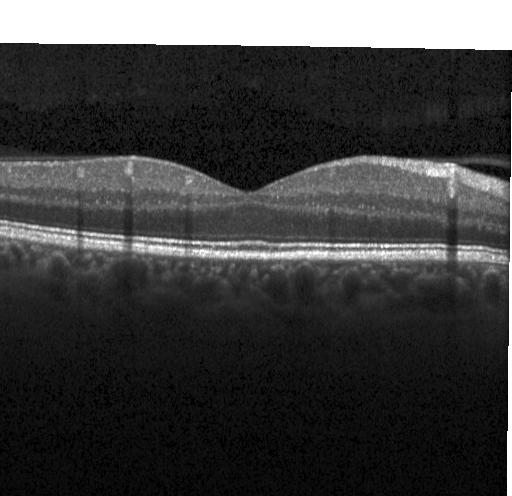
Optical coherence tomography scan · instrument: Heidelberg Spectralis · through the macula · spectral-domain OCT. Assessment: neither CNV, DME, nor drusen.